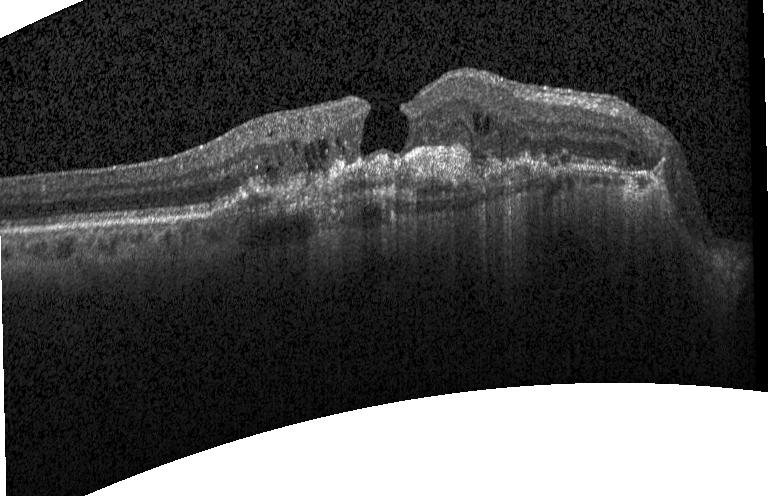

Retinal OCT B-scan; instrument: Heidelberg Spectralis; SD-OCT; through the macula. A choroidal neovascular membrane.